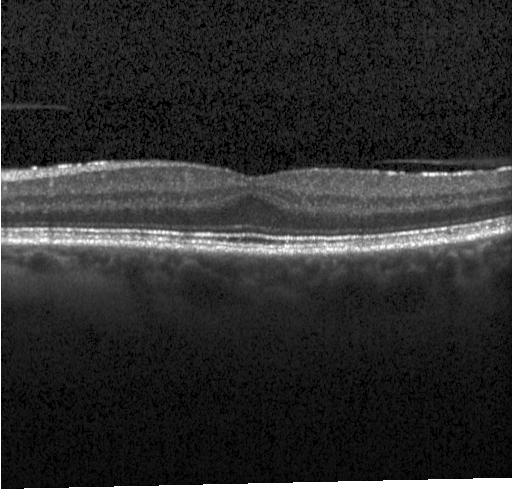 Acquired on a Heidelberg Spectralis, retinal OCT B-scan. Finding: no choroidal neovascularization, diabetic macular edema, or drusen.